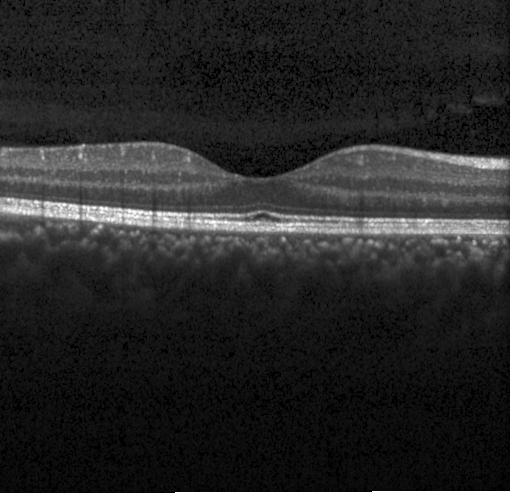 Neither choroidal neovascularization, diabetic macular edema, nor drusen.